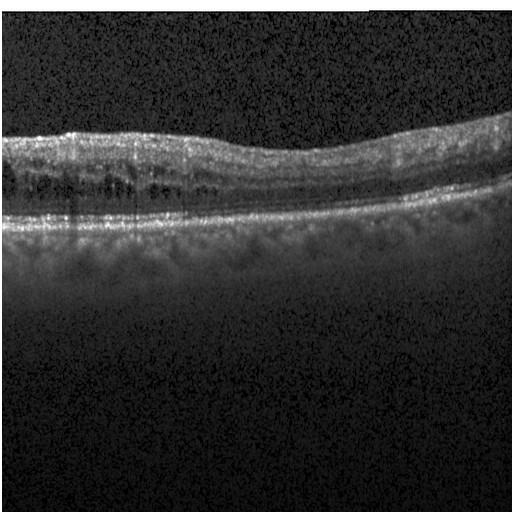

Impression: diabetic macular edema.